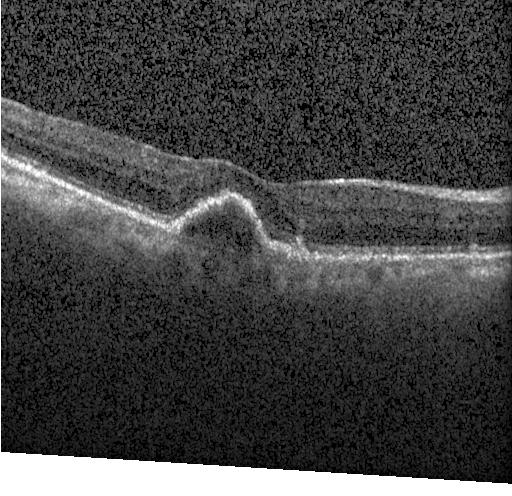
This B-scan demonstrates a choroidal neovascular membrane.